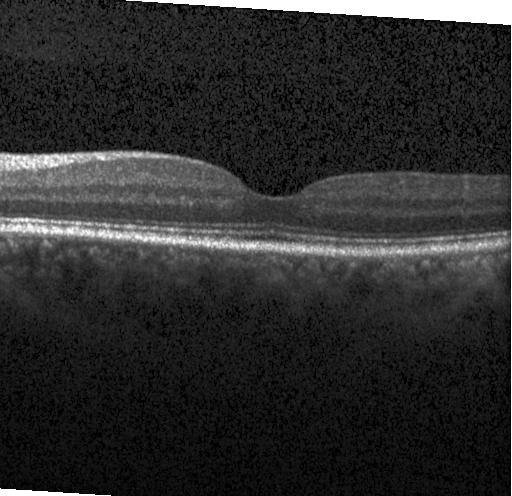

Optical coherence tomography scan — Impression: no choroidal neovascularization, diabetic macular edema, or drusen.